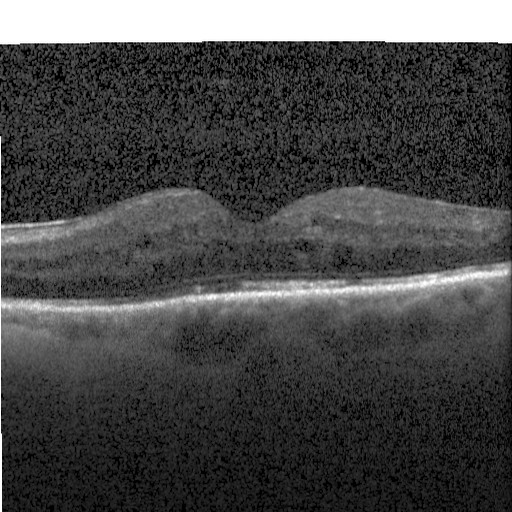 OCT finding: DME.